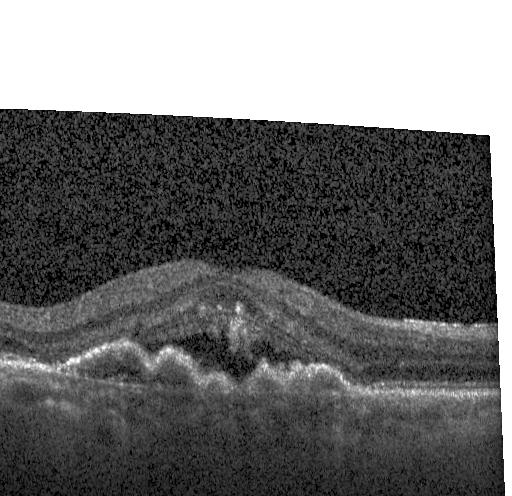 Dx: choroidal neovascularization.